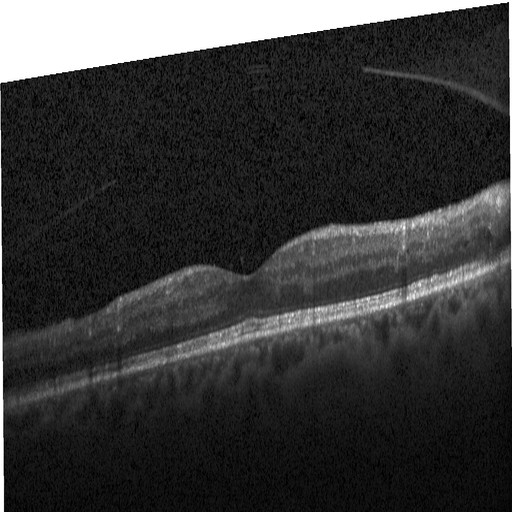
Diagnosis: DME.